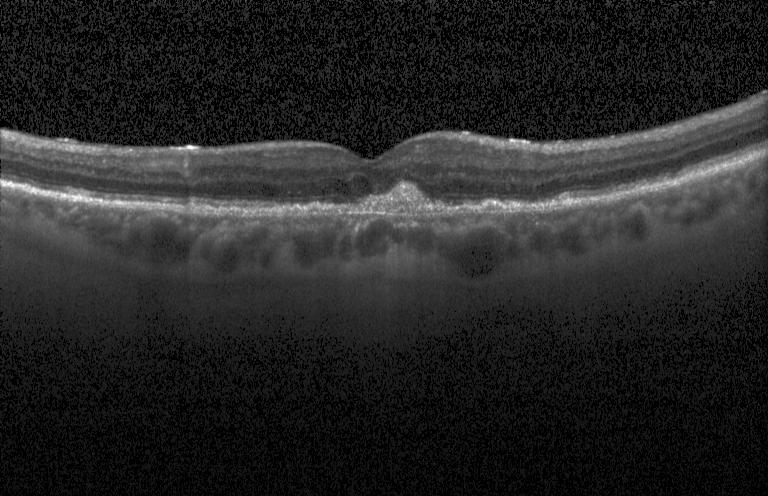 Impression: CNV.